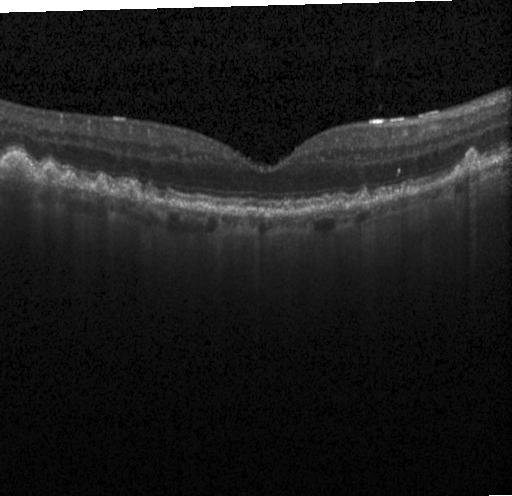 Optical coherence tomography B-scan, fovea-centered, spectral-domain OCT. Diagnosis: drusen.